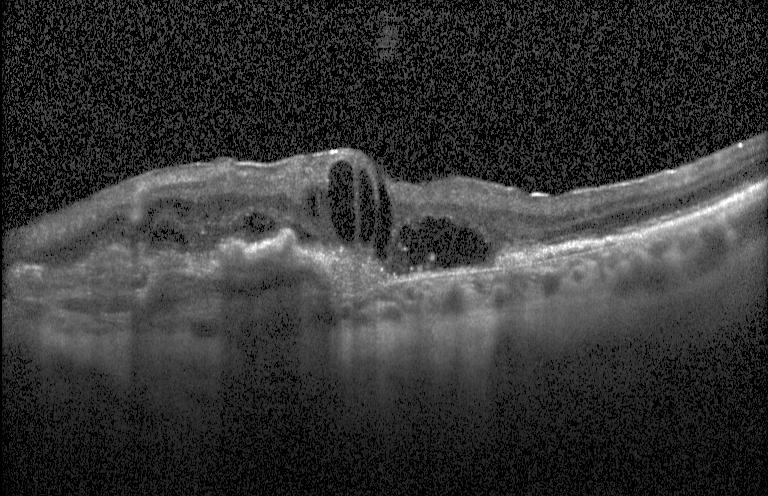 Spectral-domain OCT · optical coherence tomography B-scan
Assessment: choroidal neovascularization.